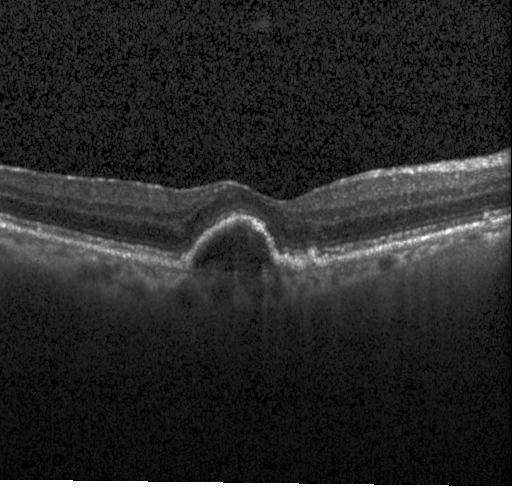

A choroidal neovascular membrane.